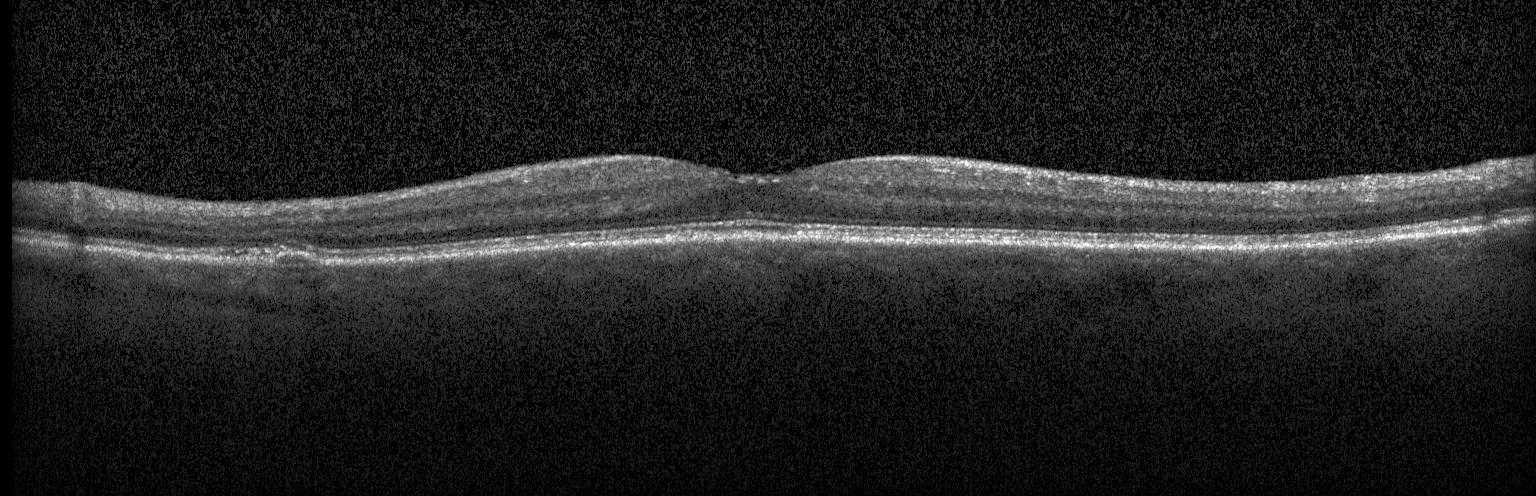
Retinal OCT cross-section showing choroidal neovascularization.